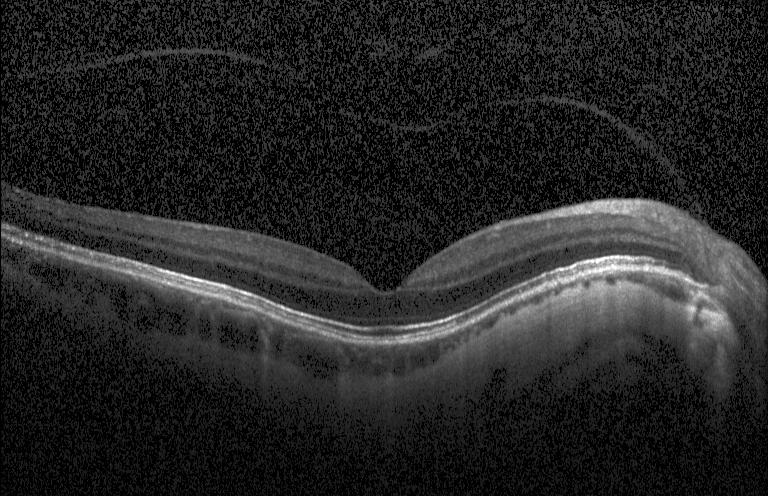
Retinal OCT B-scan. Spectral-domain optical coherence tomography.
Finding: no evidence of choroidal neovascularization, diabetic macular edema, or drusen.